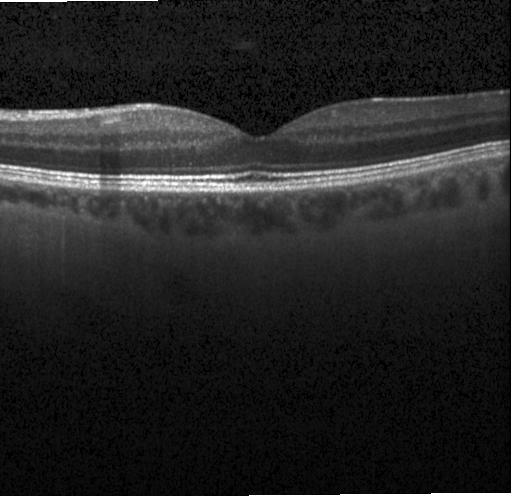 Retinal OCT B-scan · acquired on a Heidelberg Spectralis · spectral-domain optical coherence tomography. Macular OCT: no evidence of choroidal neovascularization, diabetic macular edema, or drusen.